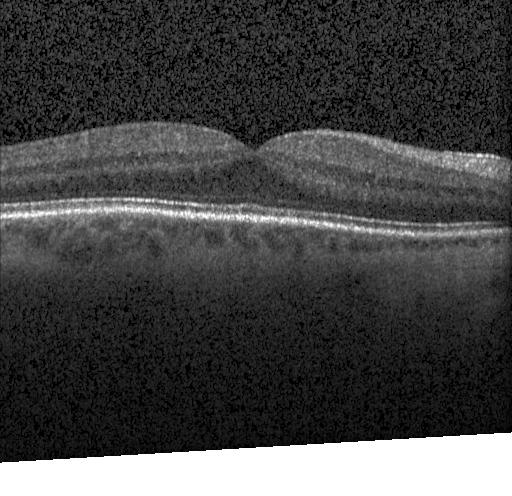
Impression: no CNV, no DME, and no drusen.